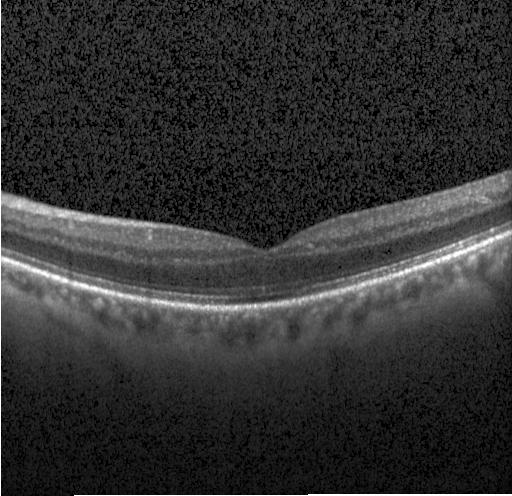
Optical coherence tomography scan
No CNV, DME, or drusen.